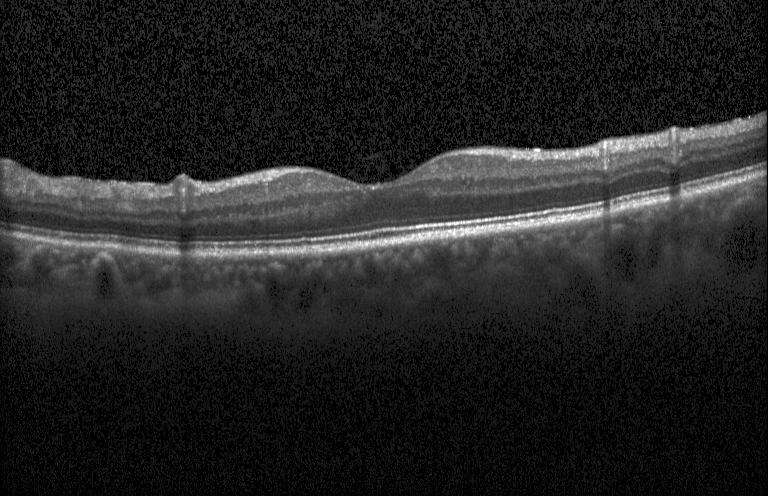
Finding: neither CNV, DME, nor drusen.